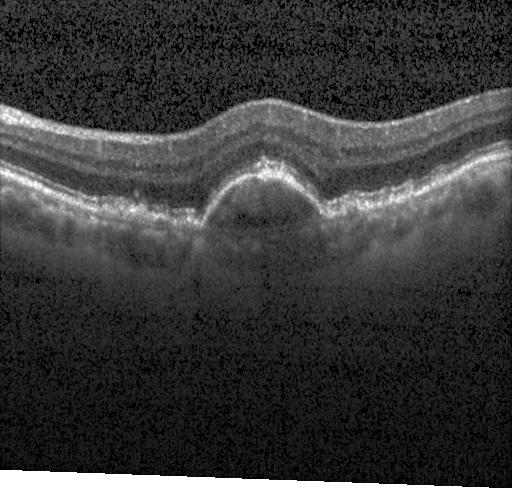 Spectral-domain optical coherence tomography · retinal OCT B-scan
OCT finding: multiple drusen.